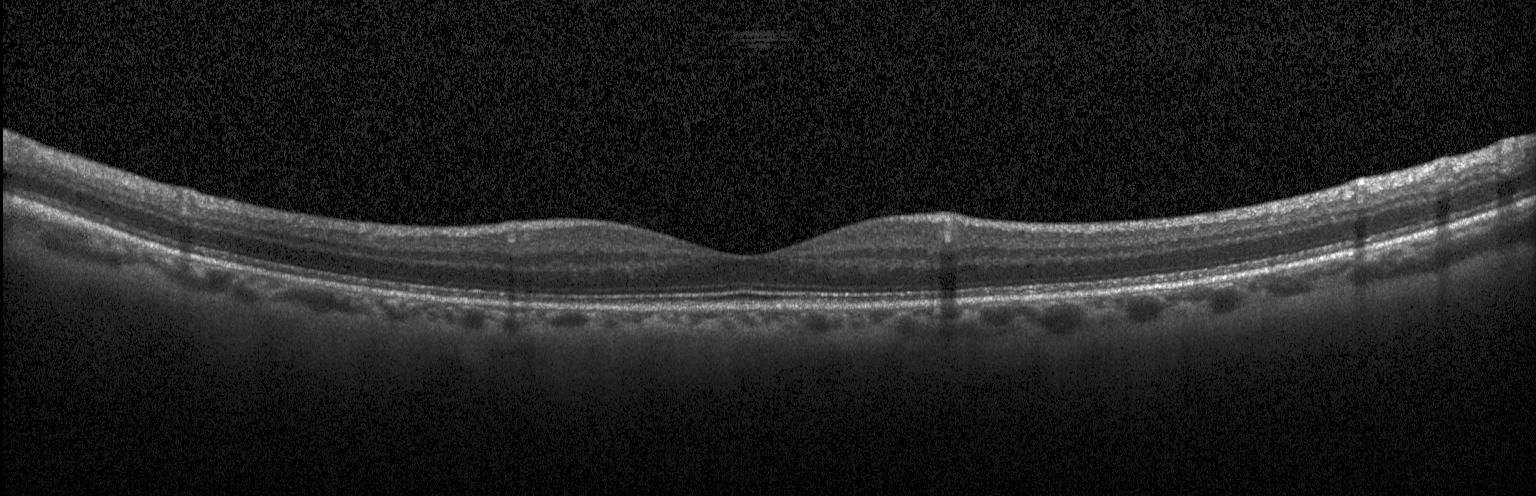

The scan shows no evidence of choroidal neovascularization, diabetic macular edema, or drusen.